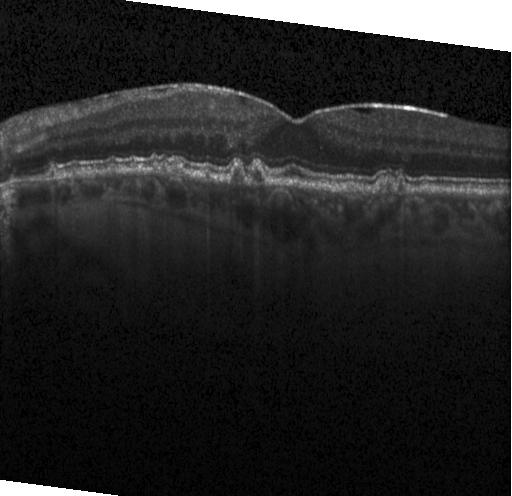 The scan shows sub-RPE drusenoid deposits.